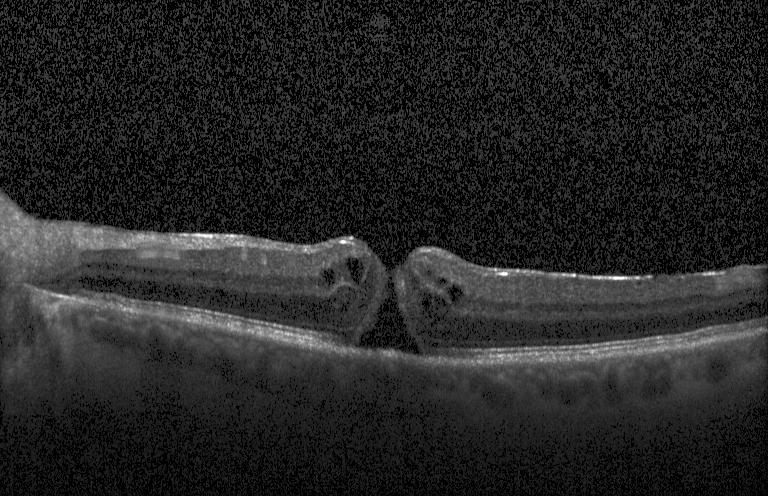 Fovea-centered; acquired on a Heidelberg Spectralis; optical coherence tomography B-scan
Impression: DME.